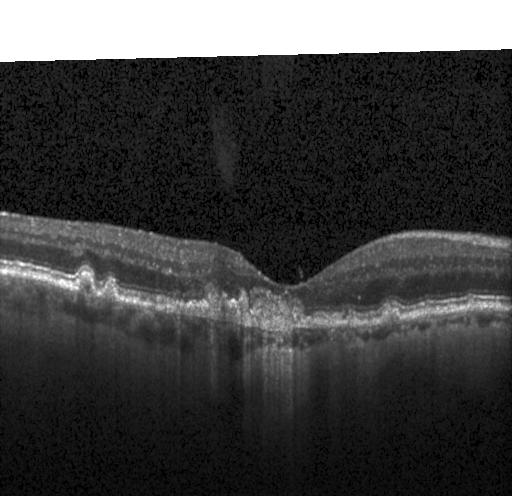
Retinal OCT B-scan. SD-OCT — Diagnosis: a choroidal neovascular membrane.